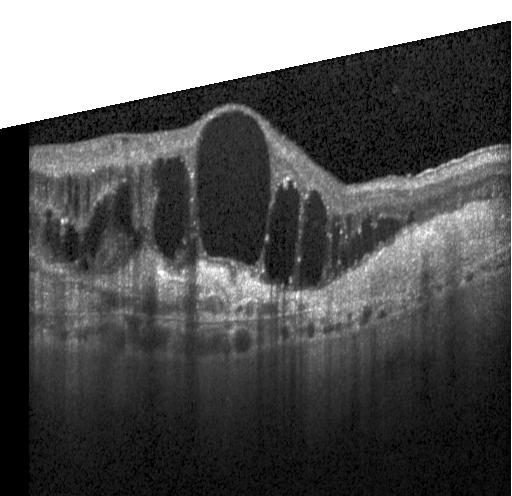

OCT line scan, spectral-domain optical coherence tomography — Choroidal neovascularization.